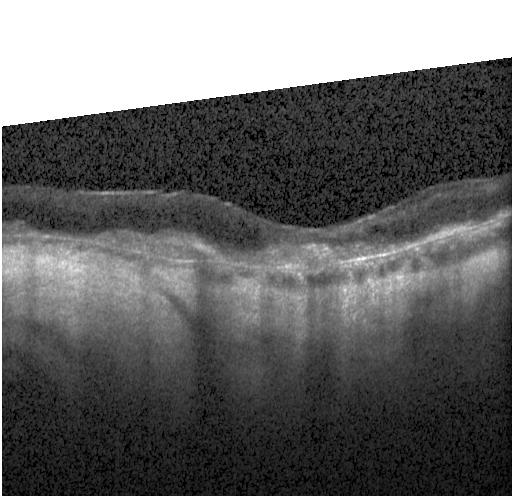
Diagnosis: a choroidal neovascular membrane.